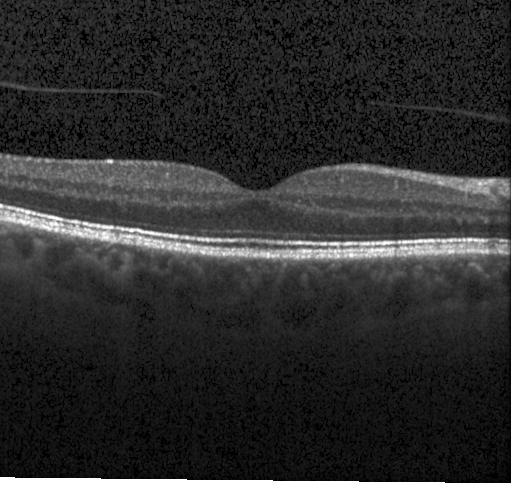
Fovea-centered, optical coherence tomography B-scan, spectral-domain optical coherence tomography, instrument: Heidelberg Spectralis — Diagnosis: neither choroidal neovascularization, diabetic macular edema, nor drusen.